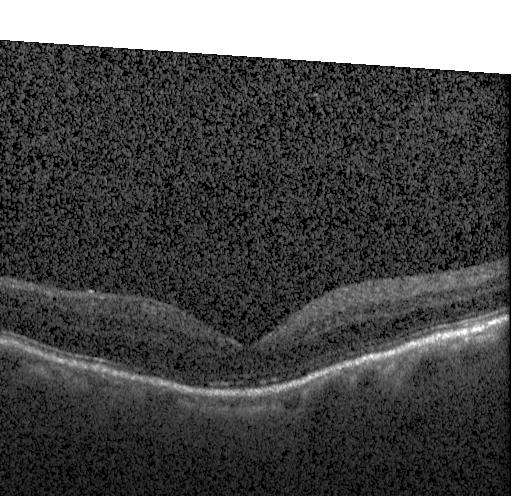

Spectral-domain optical coherence tomography, OCT B-scan, acquired on a Heidelberg Spectralis.
The scan shows neither CNV, DME, nor drusen.